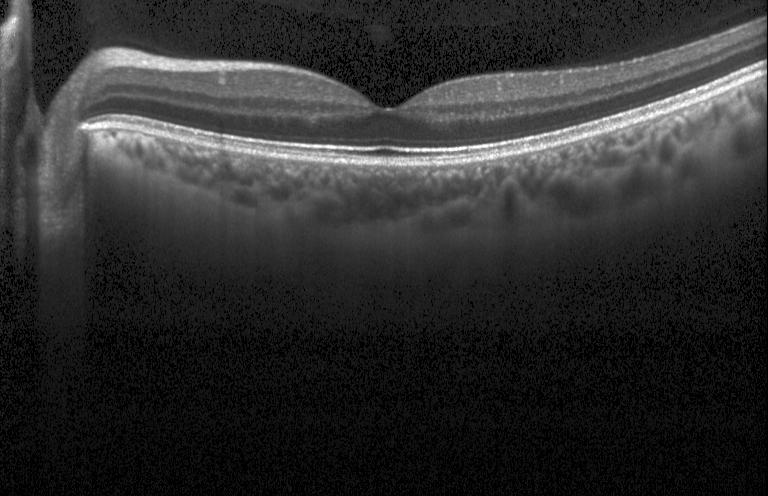 Optical coherence tomography B-scan; spectral-domain optical coherence tomography.
Finding: no choroidal neovascularization, diabetic macular edema, or drusen.